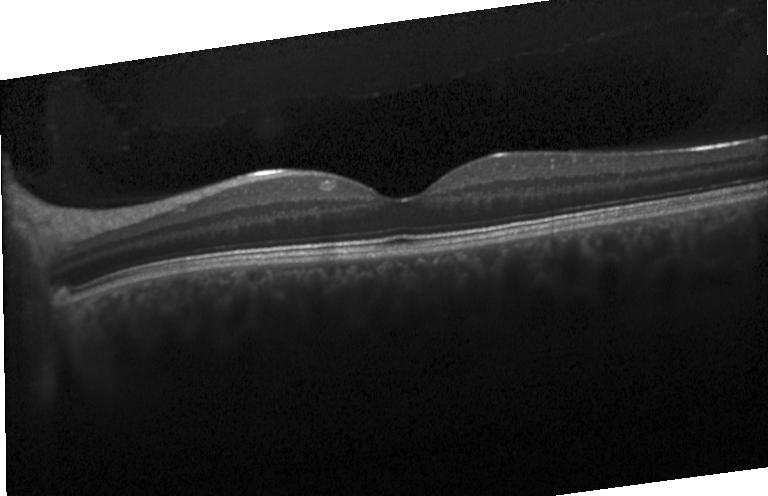

Retinal OCT B-scan; spectral-domain optical coherence tomography; macular scan; acquired on a Heidelberg Spectralis — Diagnosis: no CNV, DME, or drusen.